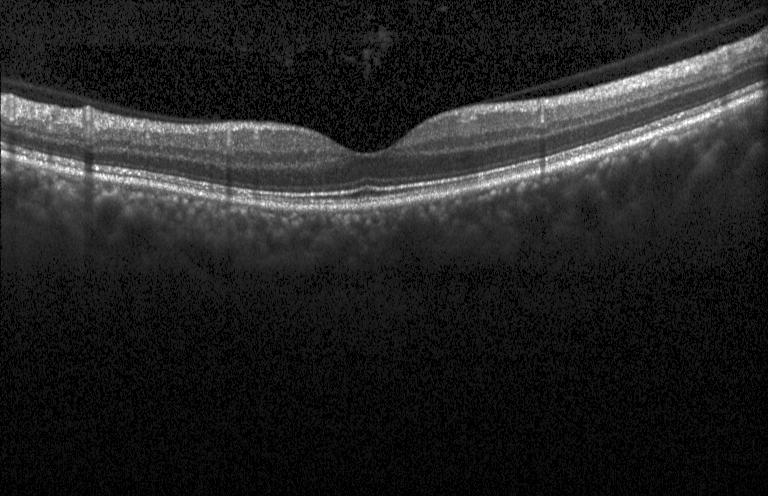
Impression: no evidence of choroidal neovascularization, diabetic macular edema, or drusen.